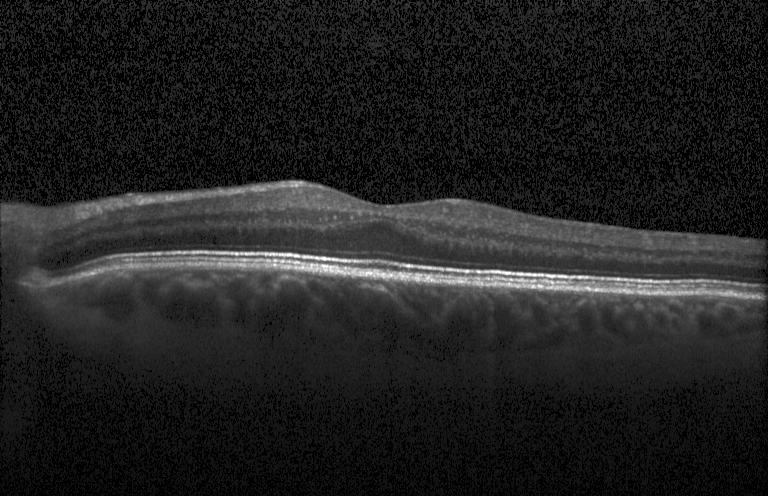

SD-OCT. Optical coherence tomography scan — OCT finding: neither CNV, DME, nor drusen.